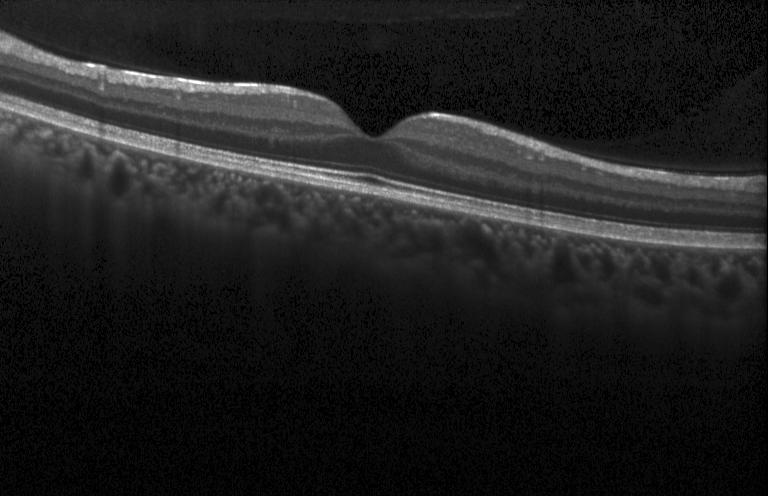

OCT line scan, acquired on a Heidelberg Spectralis, fovea-centered, SD-OCT
Impression: no evidence of choroidal neovascularization, diabetic macular edema, or drusen.